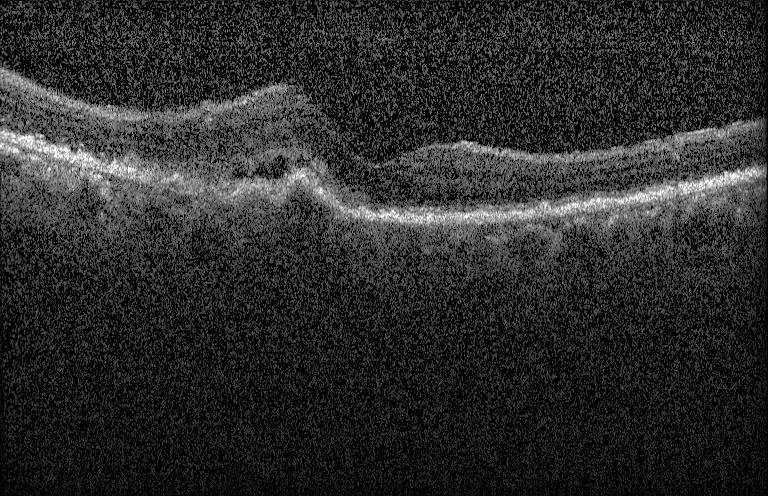
Through the macula, SD-OCT, optical coherence tomography scan. Diagnosis: a choroidal neovascular membrane.